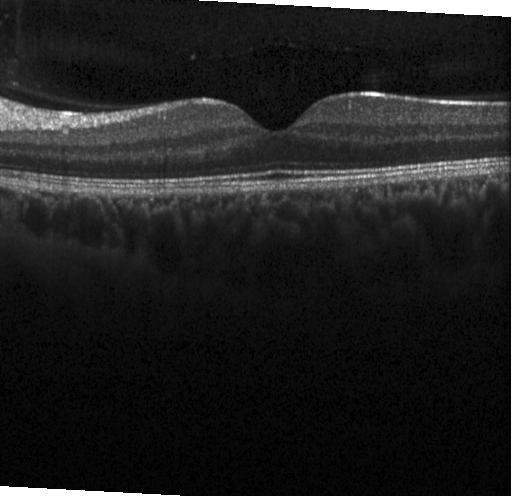

OCT finding: neither CNV, DME, nor drusen.